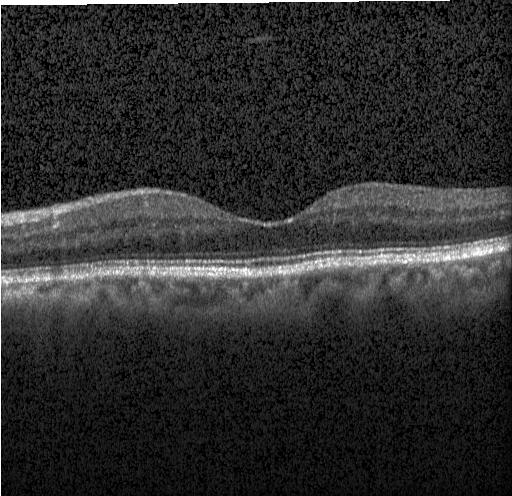 Through the macula. Heidelberg Spectralis. Retinal OCT B-scan
Impression: no choroidal neovascularization, diabetic macular edema, or drusen.